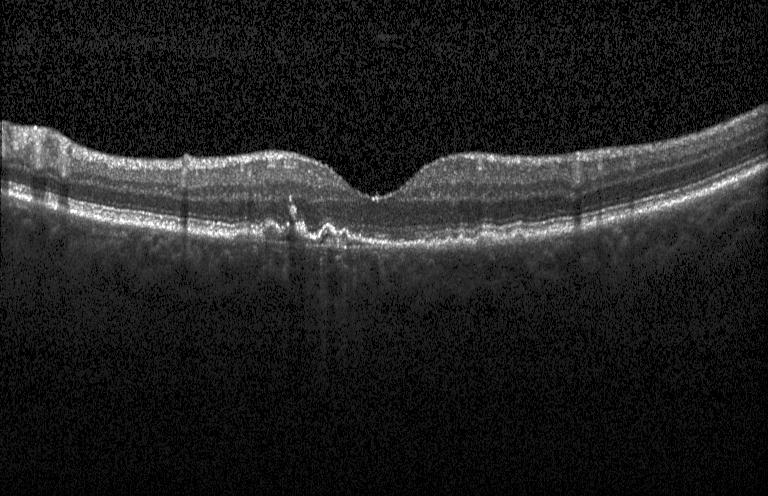
Retinal OCT cross-section — Impression: a choroidal neovascular membrane.